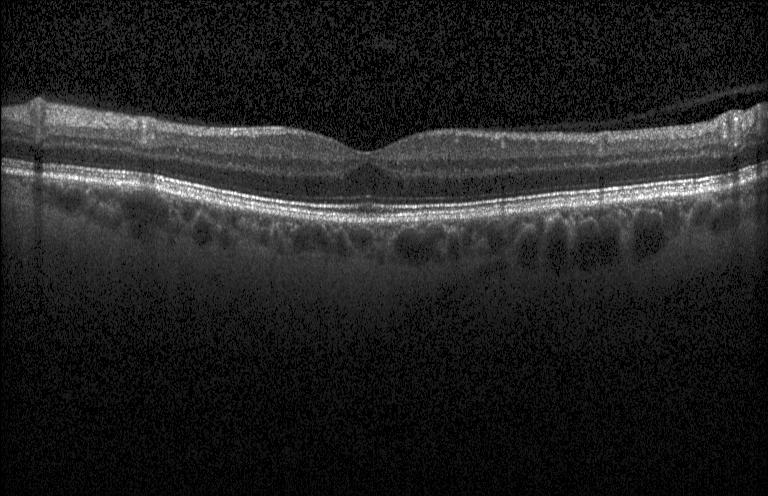

OCT line scan
No evidence of choroidal neovascularization, diabetic macular edema, or drusen.